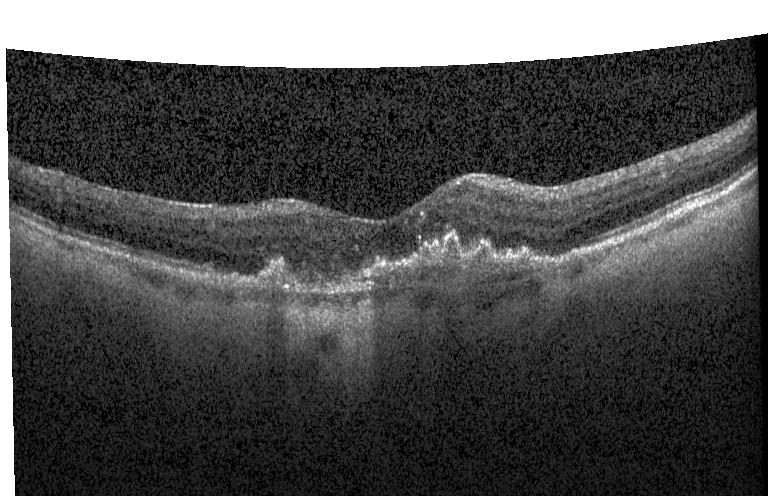
Macular OCT: a choroidal neovascular membrane.